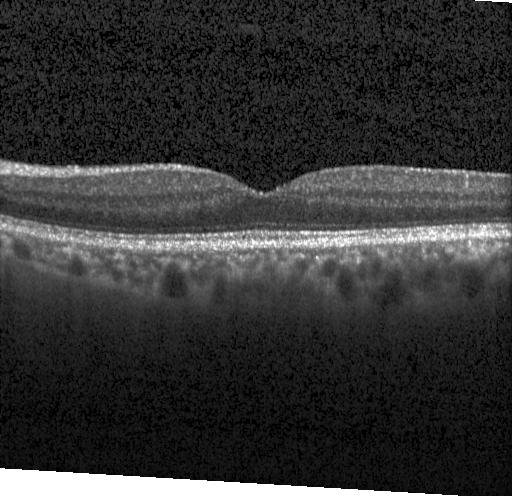

OCT B-scan. Heidelberg Spectralis
Finding: no evidence of CNV, DME, or drusen.